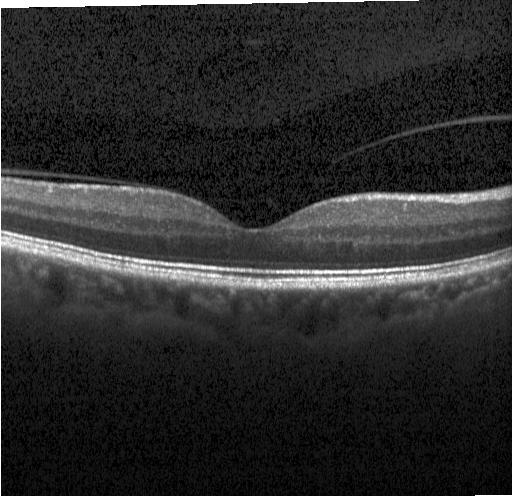 OCT finding: no choroidal neovascularization, no diabetic macular edema, and no drusen.